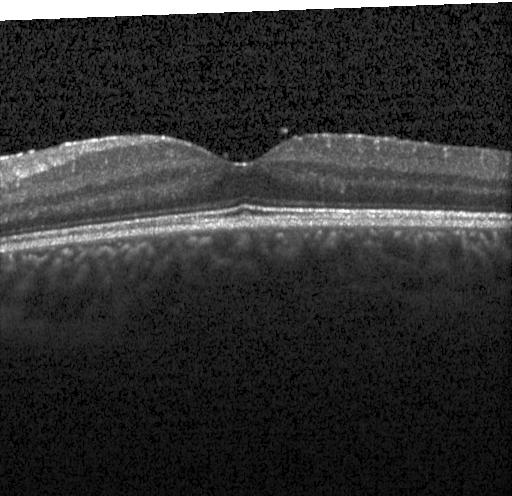

Retinal OCT cross-section. Acquired on a Heidelberg Spectralis. SD-OCT
Diagnosis: neither choroidal neovascularization, diabetic macular edema, nor drusen.